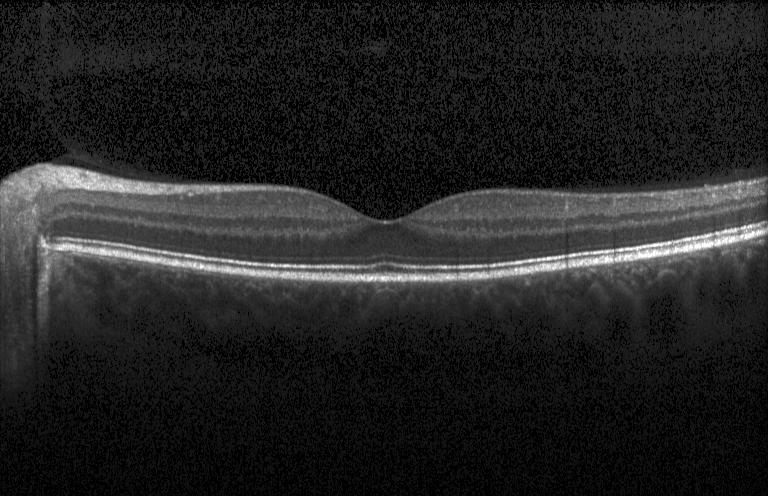
Instrument: Heidelberg Spectralis. OCT line scan.
Assessment: no choroidal neovascularization, diabetic macular edema, or drusen.